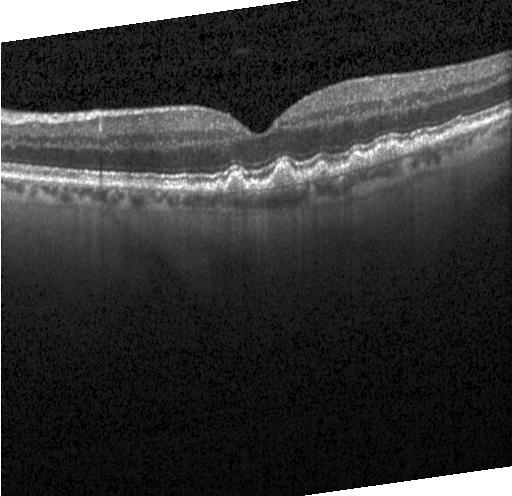 Heidelberg Spectralis, optical coherence tomography scan, spectral-domain optical coherence tomography — Impression: multiple drusen.